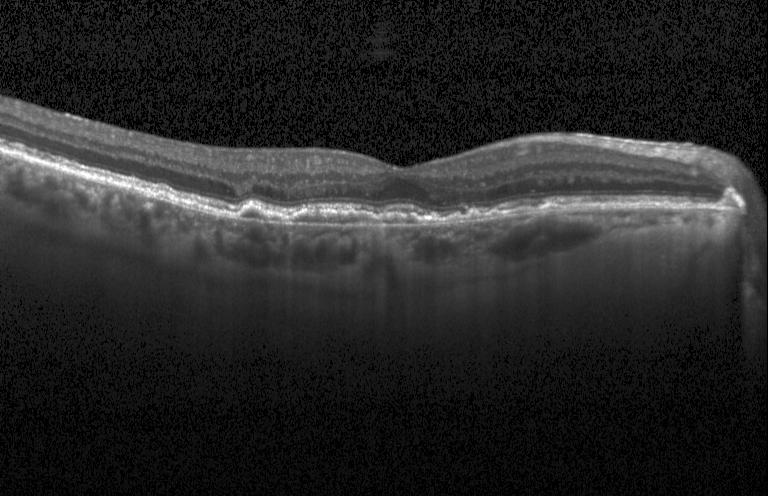 Optical coherence tomography scan. Through the macula. Heidelberg Spectralis. Assessment: a choroidal neovascular membrane.